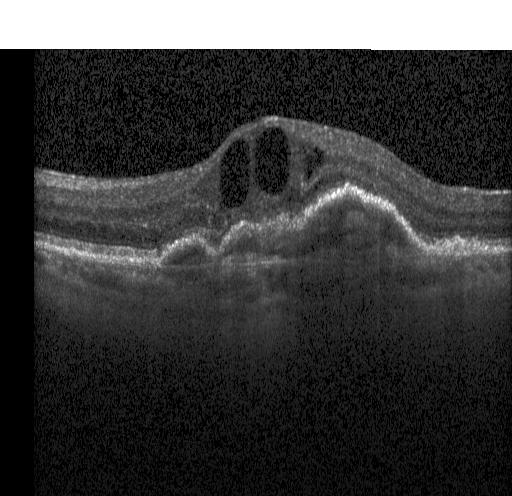
Centered on the fovea; retinal OCT B-scan; SD-OCT.
Dx: choroidal neovascularization.